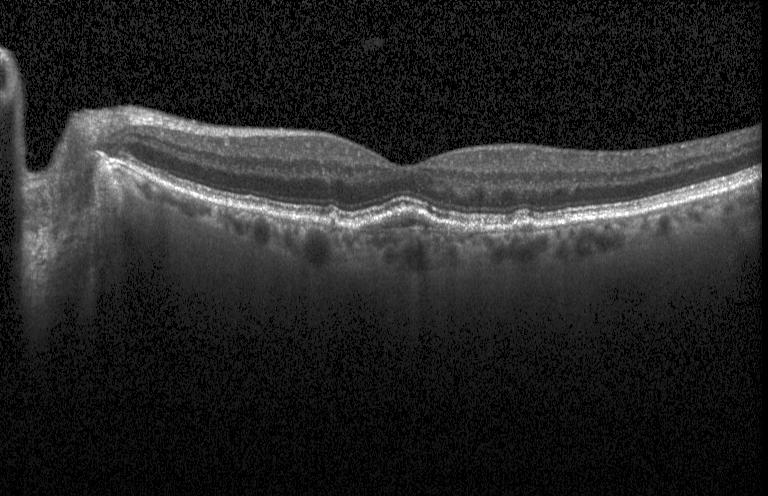 Finding: a choroidal neovascular membrane.